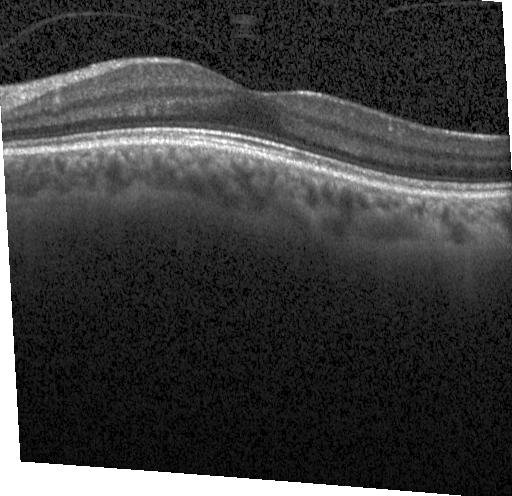 Diagnosis: no evidence of CNV, DME, or drusen.